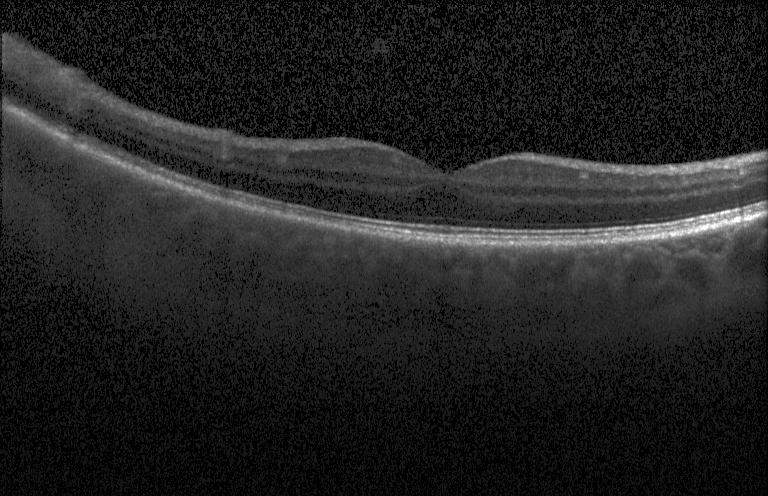
OCT B-scan, spectral-domain OCT
Diagnosis: no choroidal neovascularization, diabetic macular edema, or drusen.